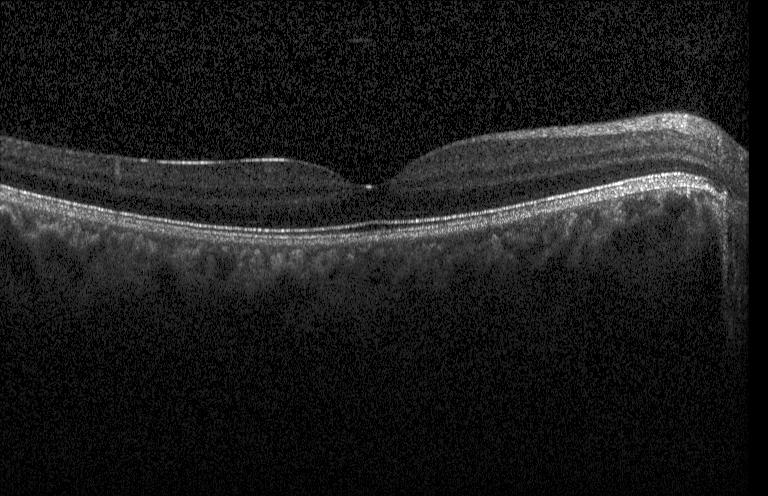 Heidelberg Spectralis OCT system; spectral-domain optical coherence tomography; horizontal scan through the fovea; retinal OCT B-scan
Diagnosis: no choroidal neovascularization, diabetic macular edema, or drusen.